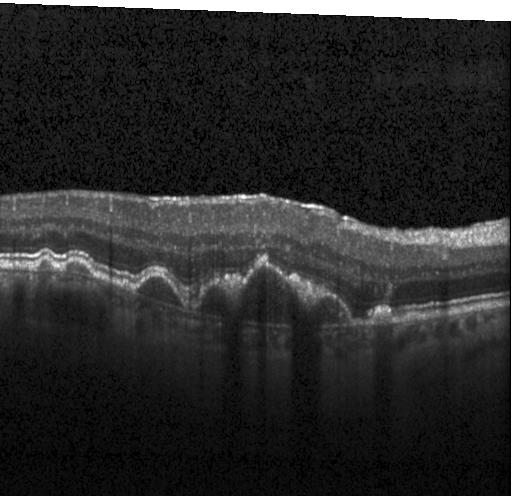

OCT B-scan showing choroidal neovascularization (CNV).